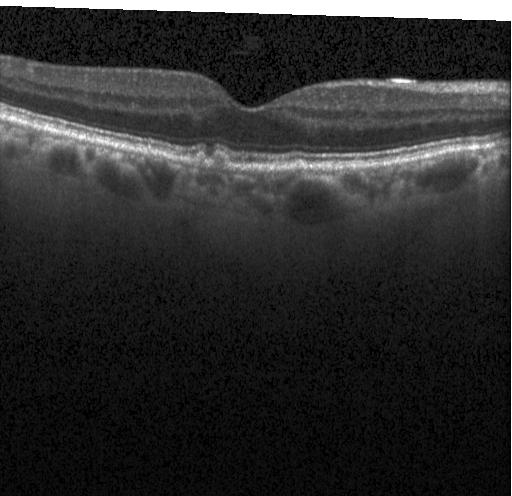 Dx: multiple drusen.